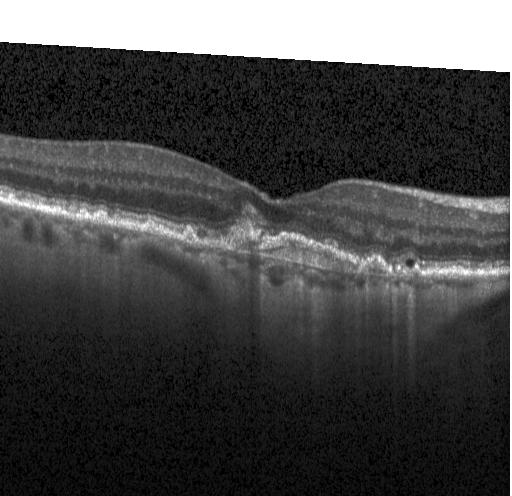
Retinal OCT B-scan, SD-OCT, through the macula, Heidelberg Spectralis — Finding: choroidal neovascularization.